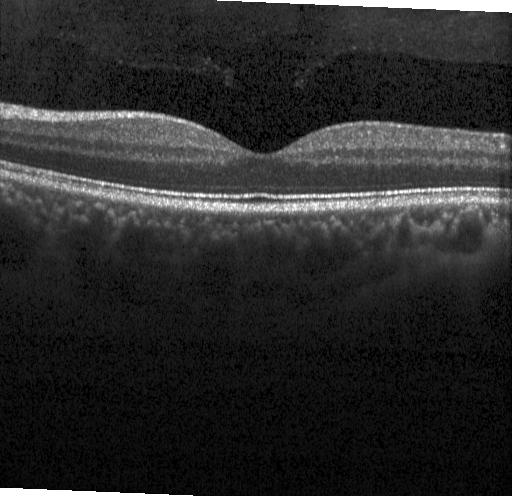
Acquired on a Heidelberg Spectralis. OCT line scan. SD-OCT.
Impression: no choroidal neovascularization, no diabetic macular edema, and no drusen.